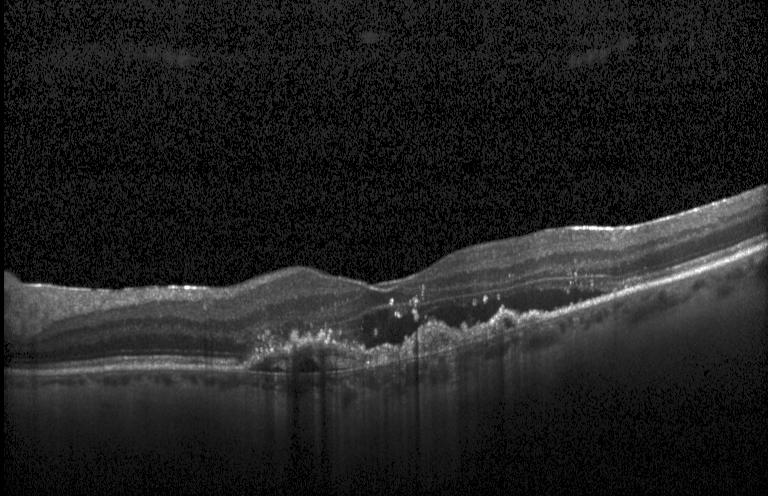 Finding: choroidal neovascularization (CNV).